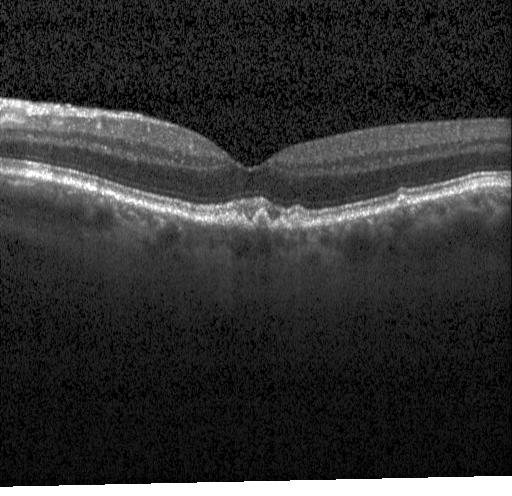

Macular OCT: multiple drusen.